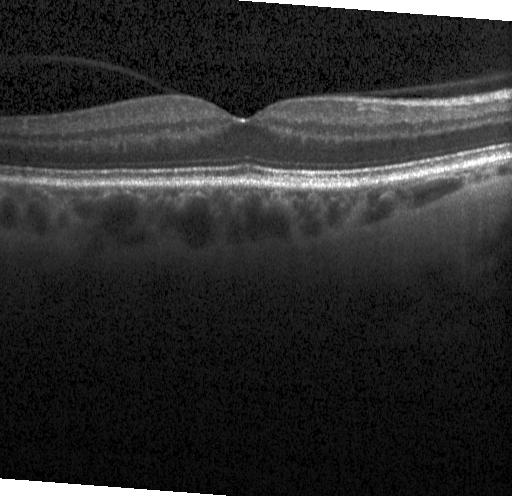 Spectral-domain OCT B-scan: no evidence of CNV, DME, or drusen.